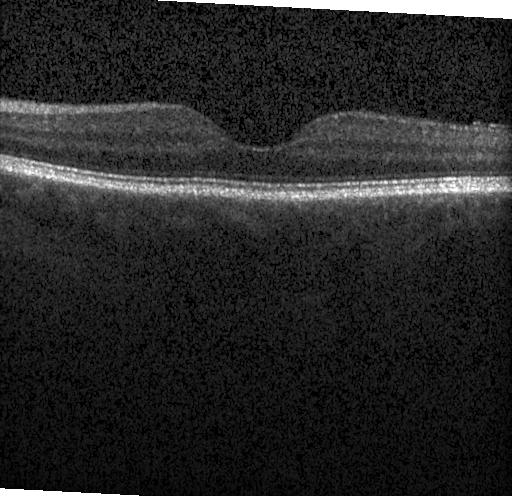 The scan shows no CNV, no DME, and no drusen.